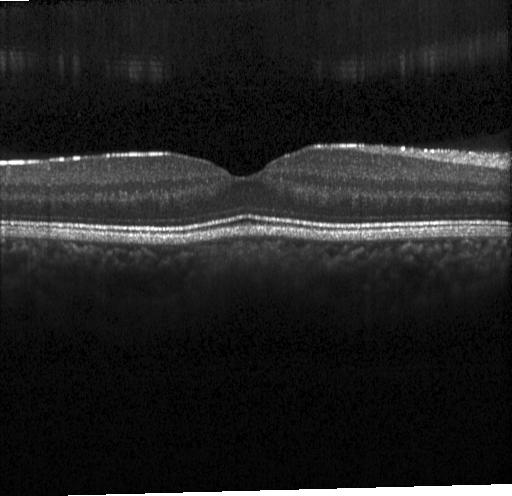
Macular OCT: no evidence of choroidal neovascularization, diabetic macular edema, or drusen.